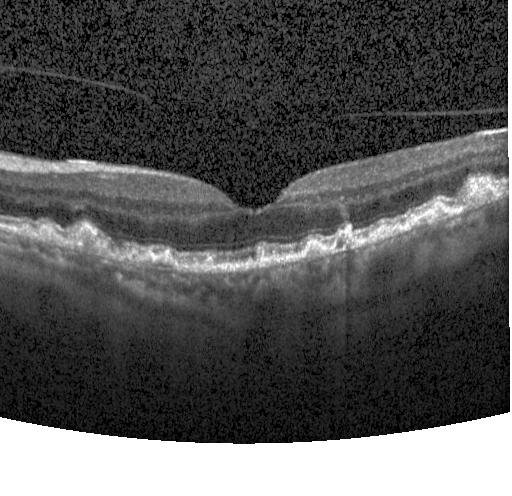

OCT line scan
Assessment: sub-RPE drusenoid deposits.